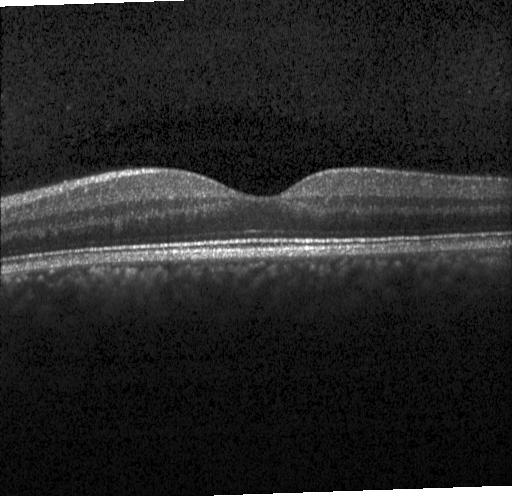
Retinal OCT B-scan · horizontal scan through the fovea · instrument: Heidelberg Spectralis
No evidence of CNV, DME, or drusen.